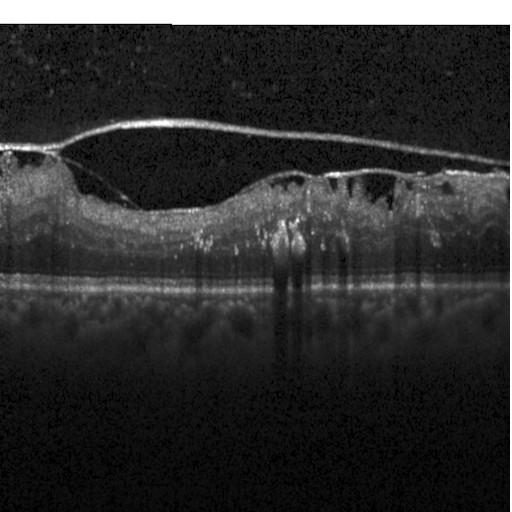
Optical coherence tomography scan. Centered on the fovea. Spectral-domain optical coherence tomography. Instrument: Heidelberg Spectralis. Diagnosis: diabetic macular edema (DME).